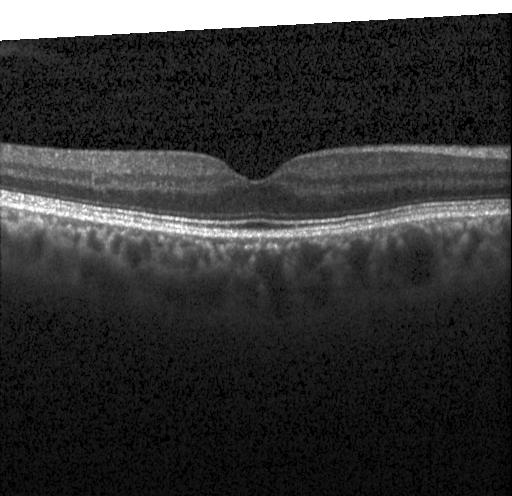

Finding: neither choroidal neovascularization, diabetic macular edema, nor drusen.